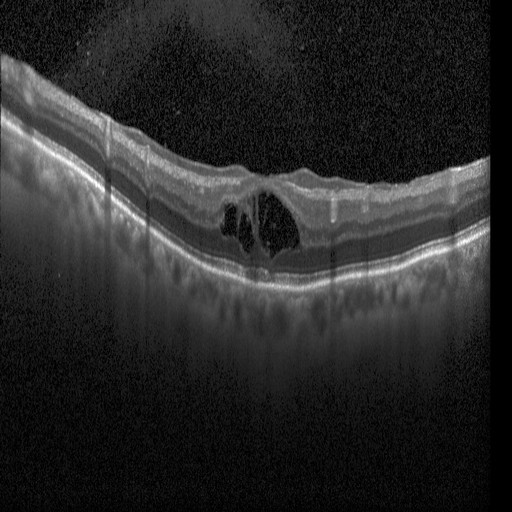

Retinal OCT B-scan · SD-OCT · through the macula
Diagnosis: diabetic macular edema.